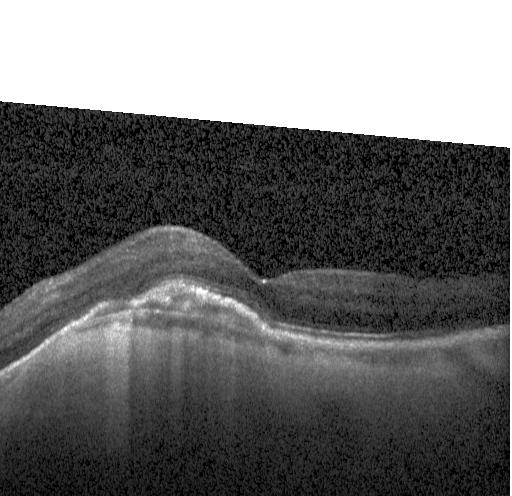 Retinal OCT cross-section showing a choroidal neovascular membrane.